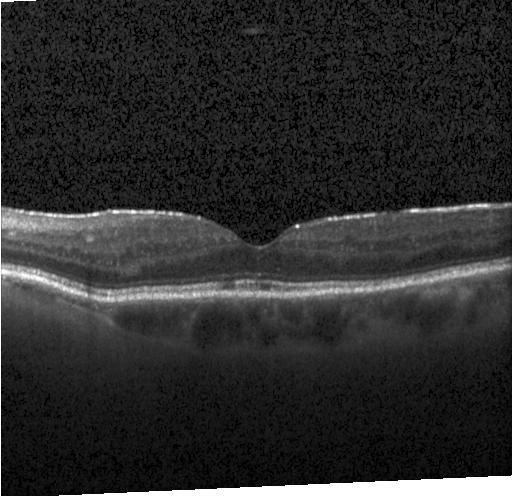 Spectral-domain OCT, OCT line scan. OCT finding: no evidence of choroidal neovascularization, diabetic macular edema, or drusen.